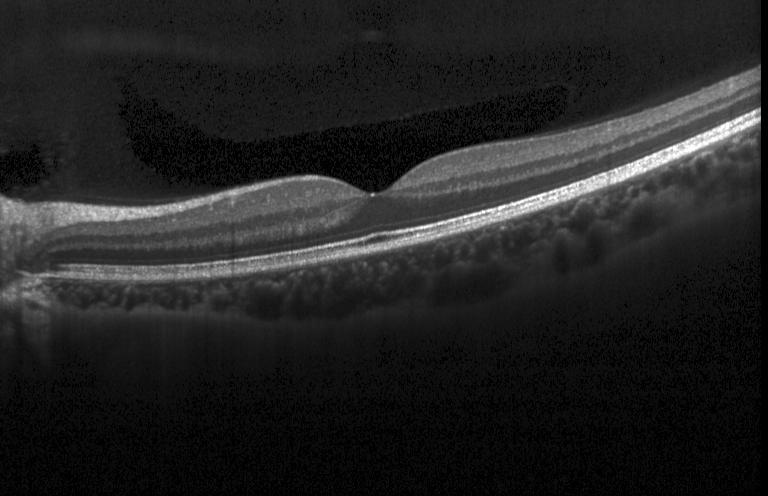
Optical coherence tomography scan.
Finding: no choroidal neovascularization, diabetic macular edema, or drusen.